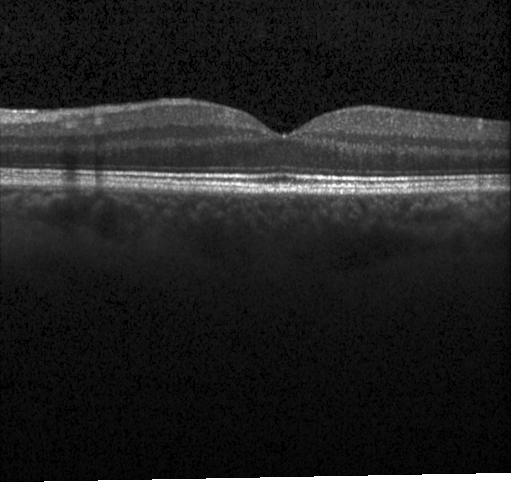 Centered on the fovea; retinal OCT B-scan
Diagnosis: neither choroidal neovascularization, diabetic macular edema, nor drusen.